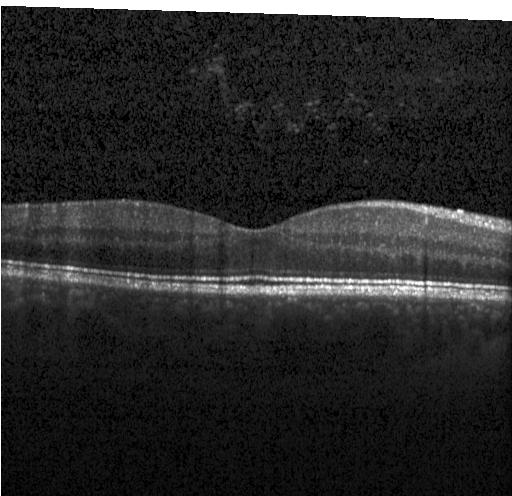 Retinal OCT cross-section showing no choroidal neovascularization, diabetic macular edema, or drusen.